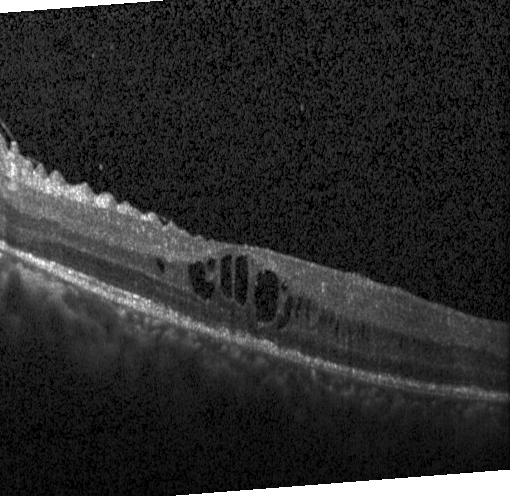 This B-scan demonstrates diabetic macular edema.